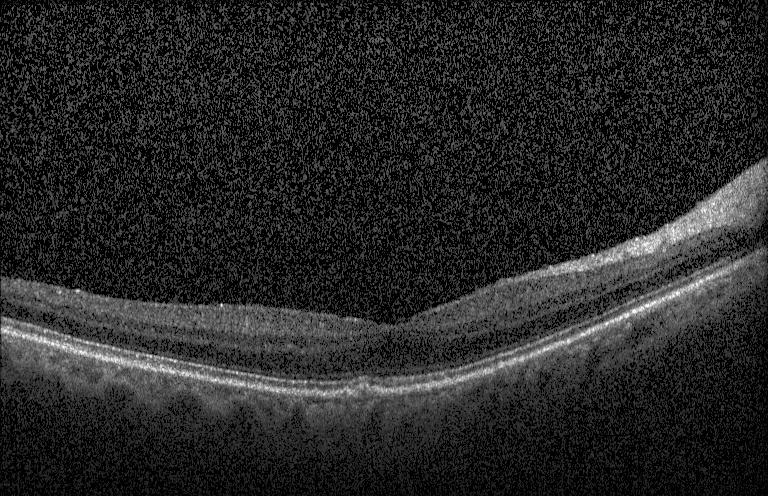
OCT scan showing drusen.